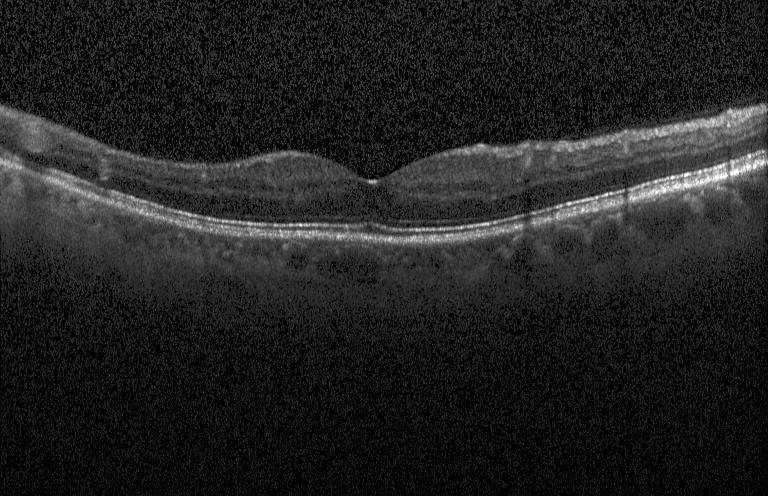 OCT B-scan showing no evidence of choroidal neovascularization, diabetic macular edema, or drusen.